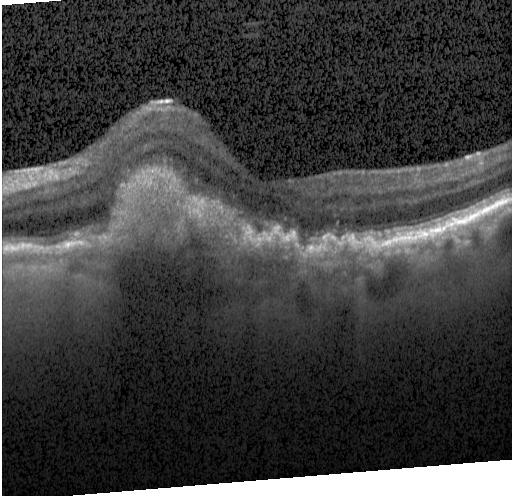
Finding: choroidal neovascularization.